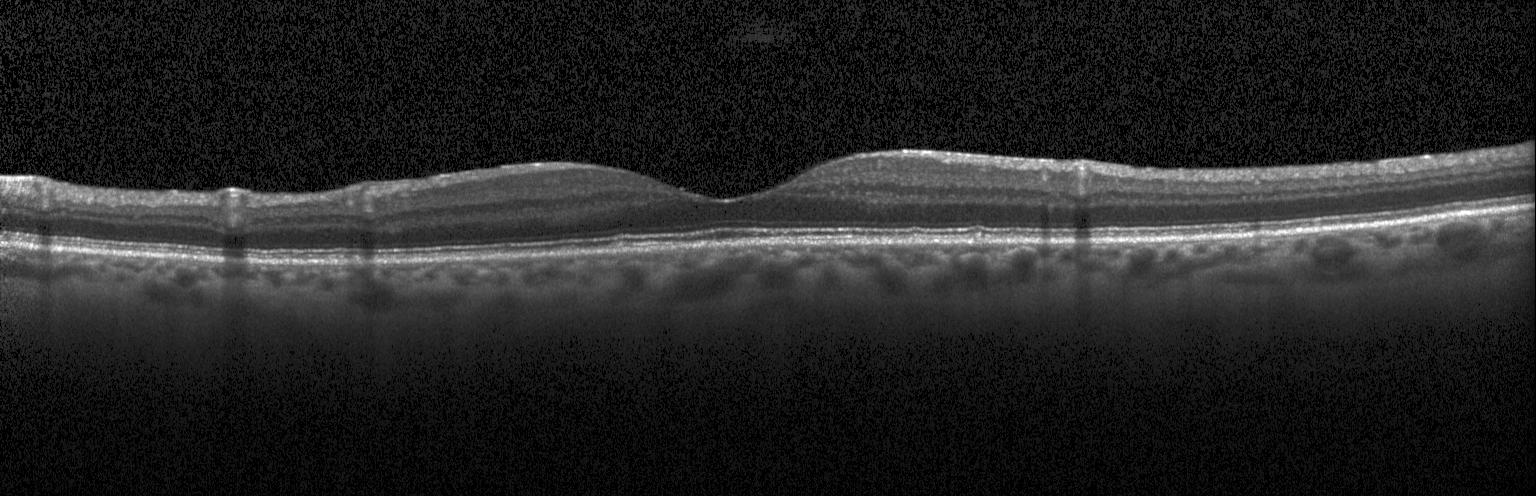 This B-scan demonstrates neither choroidal neovascularization, diabetic macular edema, nor drusen.